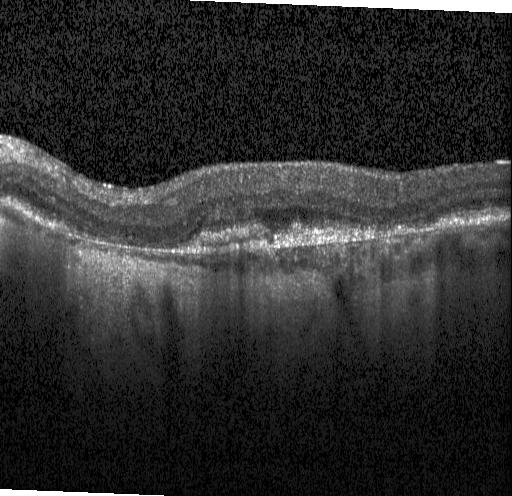
OCT line scan. Macular scan. Instrument: Heidelberg Spectralis. SD-OCT.
Choroidal neovascularization.